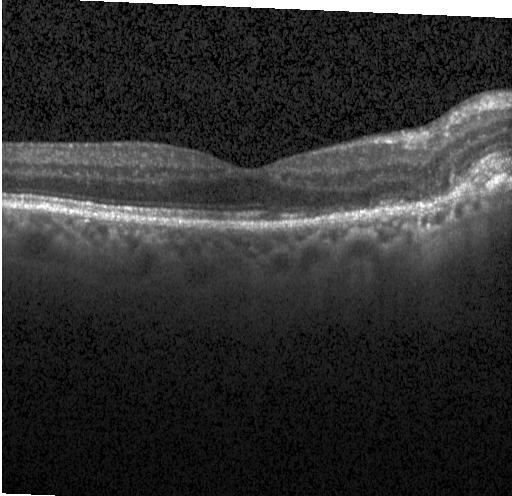

Horizontal scan through the fovea, optical coherence tomography scan, instrument: Heidelberg Spectralis. This B-scan demonstrates choroidal neovascularization (CNV).